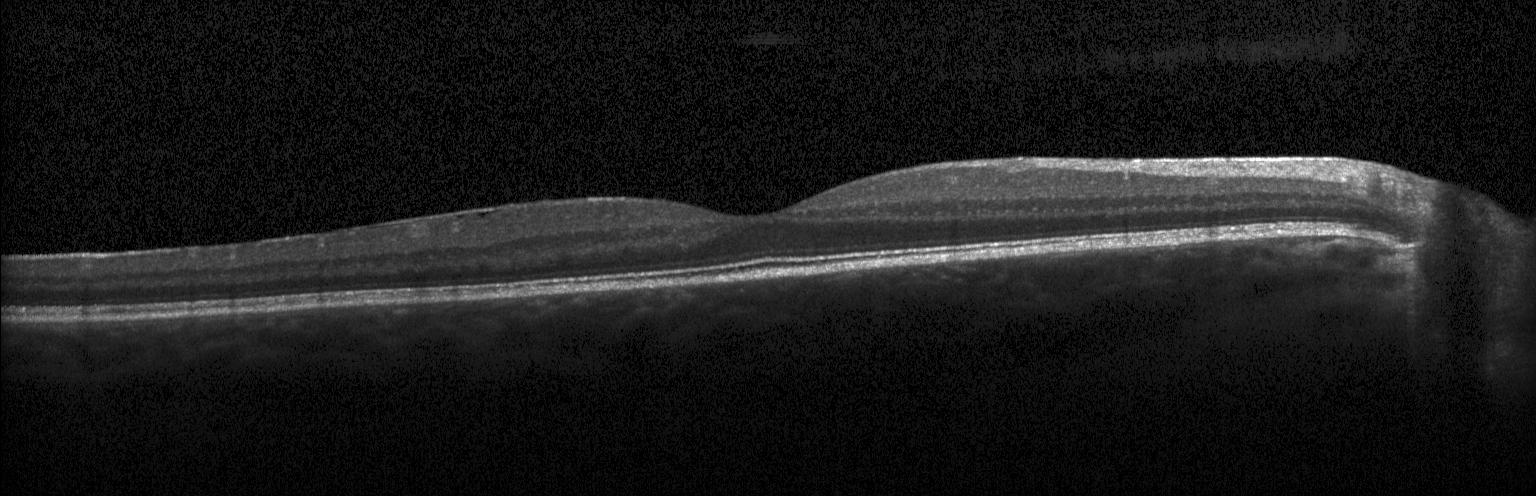
This B-scan demonstrates no evidence of CNV, DME, or drusen.